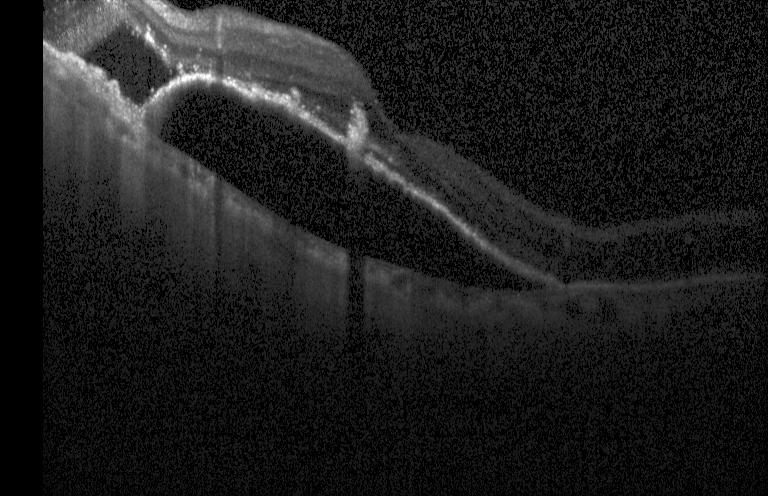
Optical coherence tomography B-scan. Acquired on a Heidelberg Spectralis. Centered on the fovea. SD-OCT. Finding: a choroidal neovascular membrane.